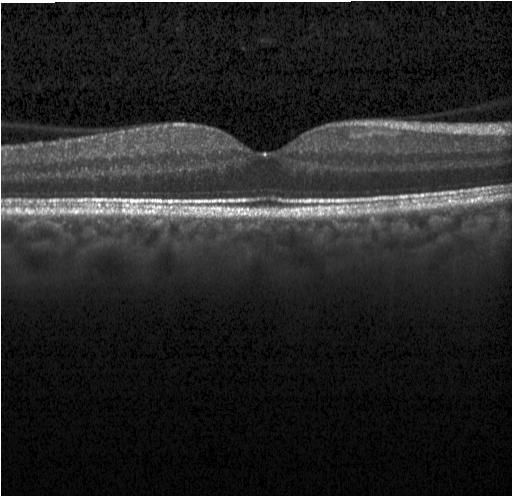
Impression: neither choroidal neovascularization, diabetic macular edema, nor drusen.